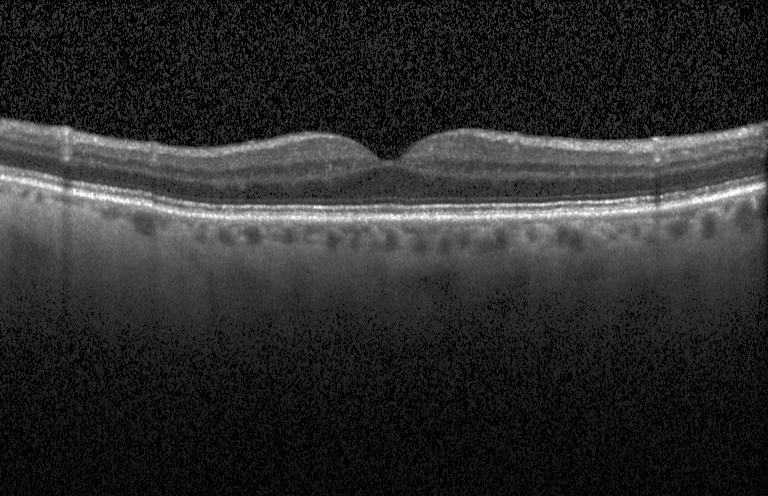

Retinal OCT B-scan
Finding: no CNV, no DME, and no drusen.